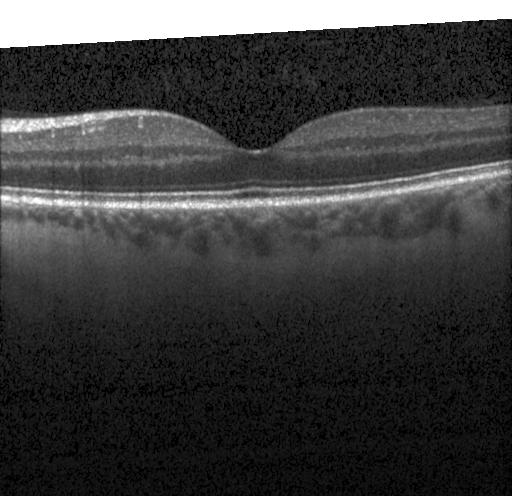
OCT B-scan — Impression: no CNV, DME, or drusen.